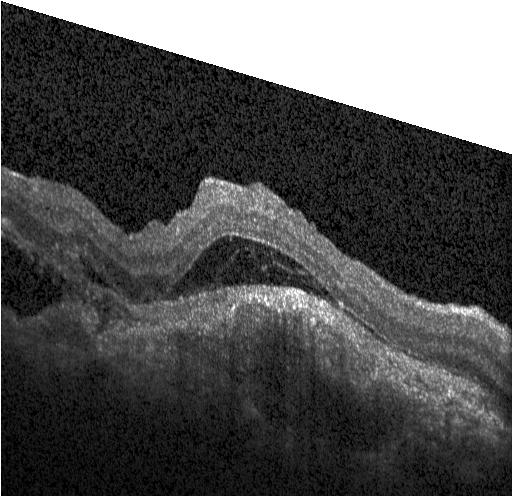

Acquired on a Heidelberg Spectralis, through the macula, retinal OCT cross-section.
Assessment: a choroidal neovascular membrane.